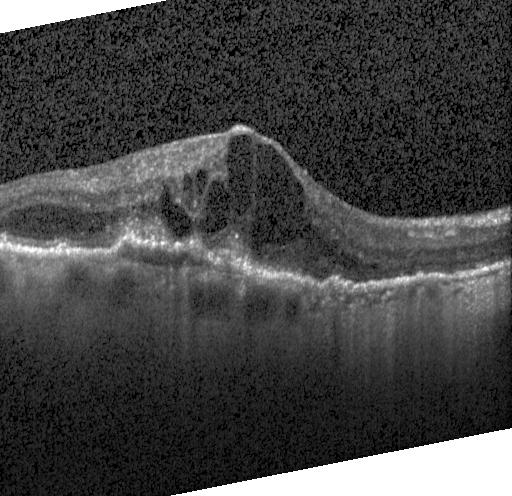
Spectral-domain optical coherence tomography · OCT line scan. Impression: a choroidal neovascular membrane.